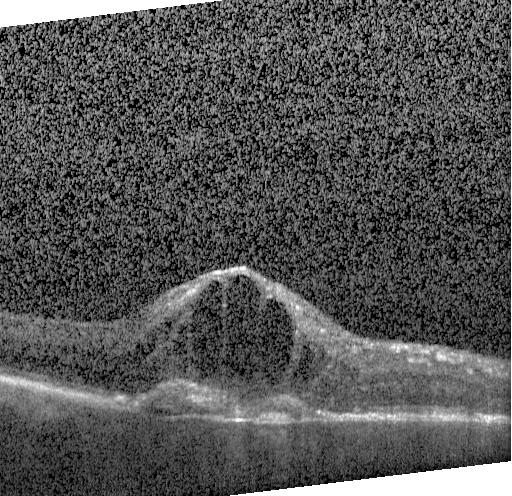 Optical coherence tomography scan — Diagnosis: a choroidal neovascular membrane.